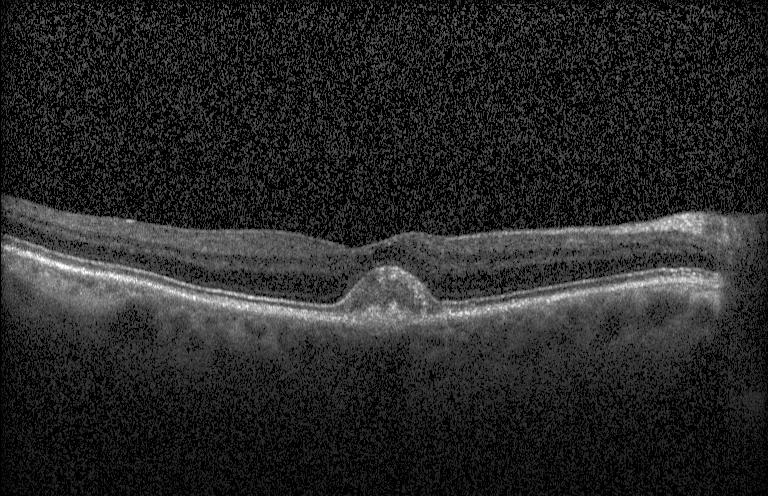

Spectral-domain OCT · OCT line scan · centered on the fovea. This B-scan demonstrates choroidal neovascularization (CNV).